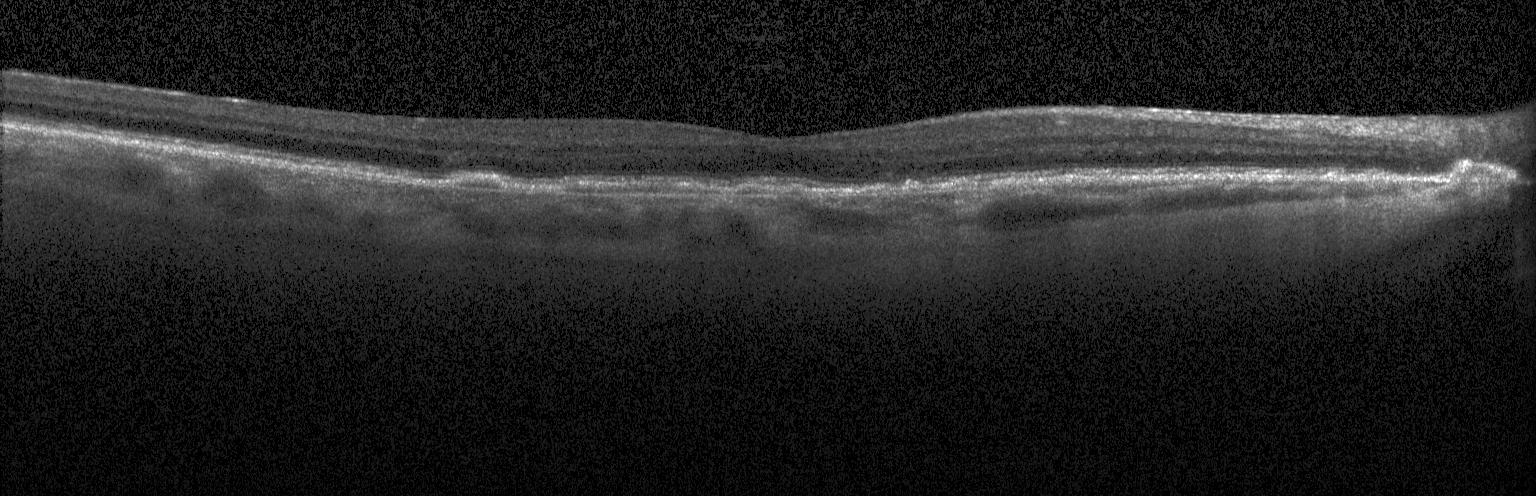 Macular scan. Optical coherence tomography B-scan. Dx: CNV.